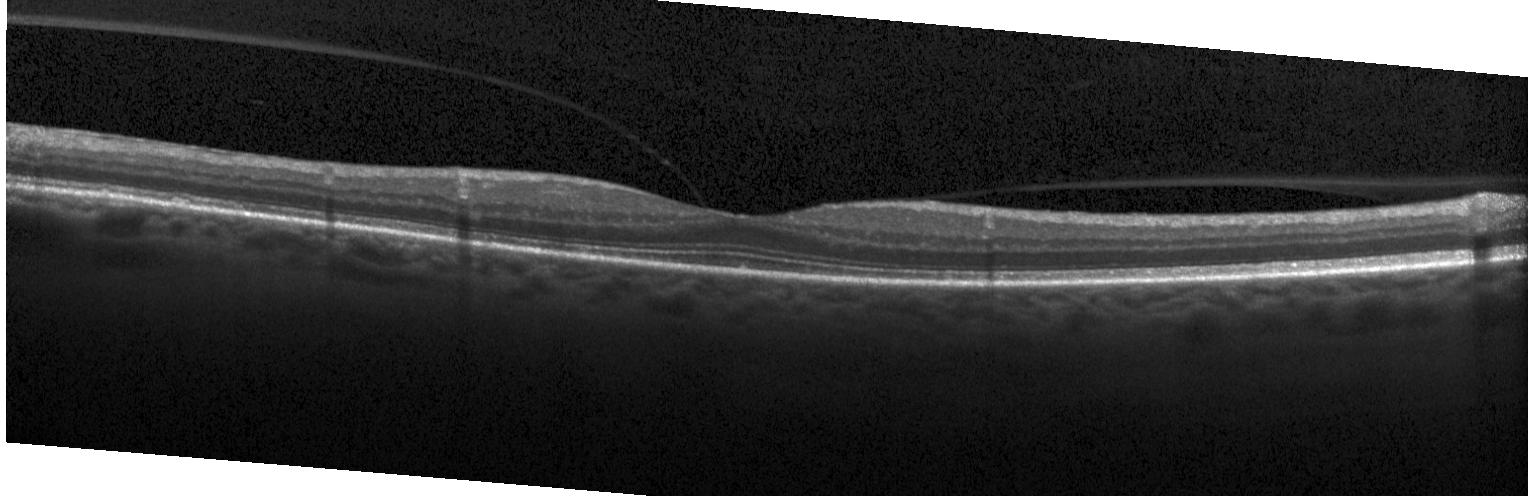 Diagnosis: no evidence of choroidal neovascularization, diabetic macular edema, or drusen.